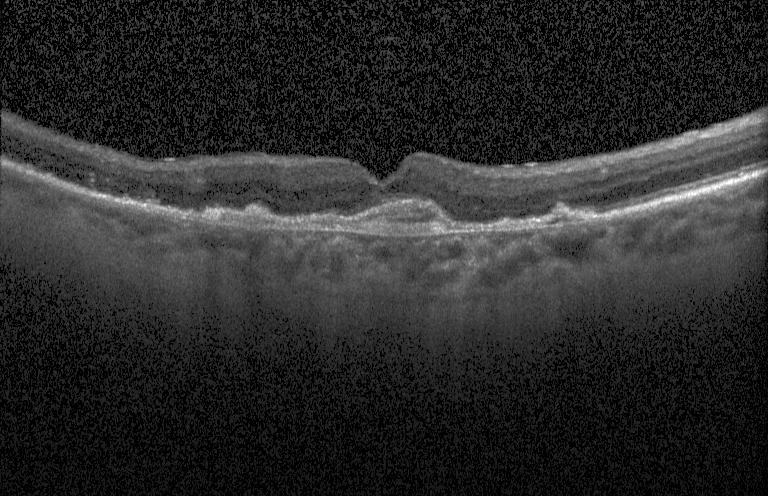 Finding: choroidal neovascularization.